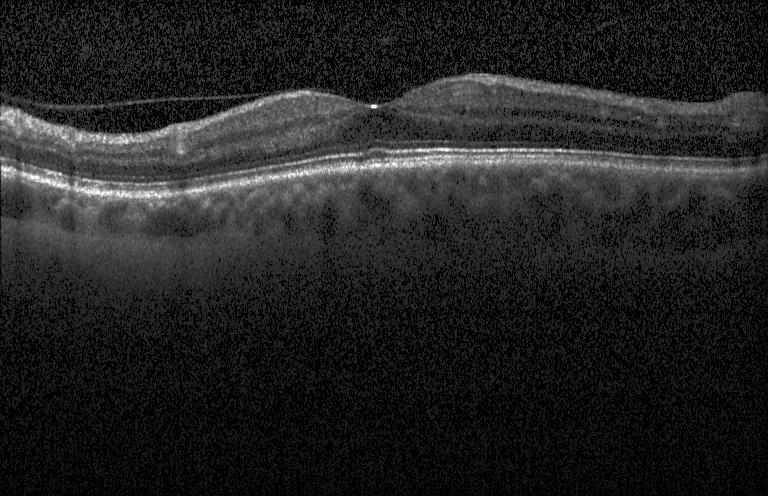
OCT B-scan — This B-scan demonstrates no evidence of choroidal neovascularization, diabetic macular edema, or drusen.